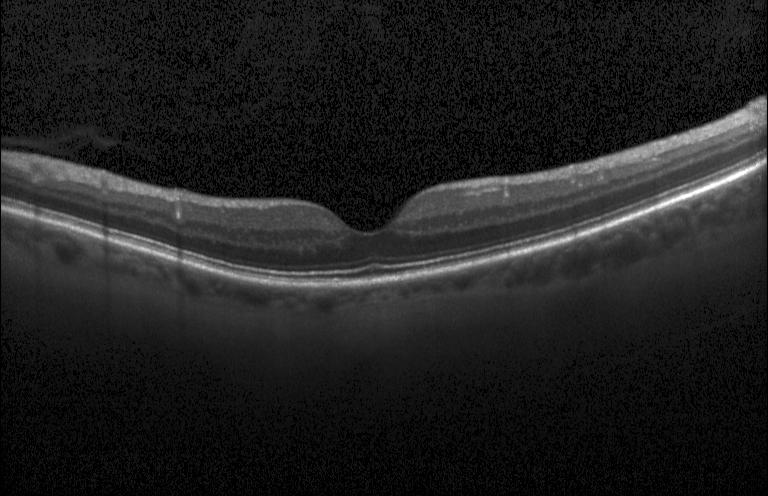
Horizontal scan through the fovea. OCT line scan. This B-scan demonstrates neither CNV, DME, nor drusen.